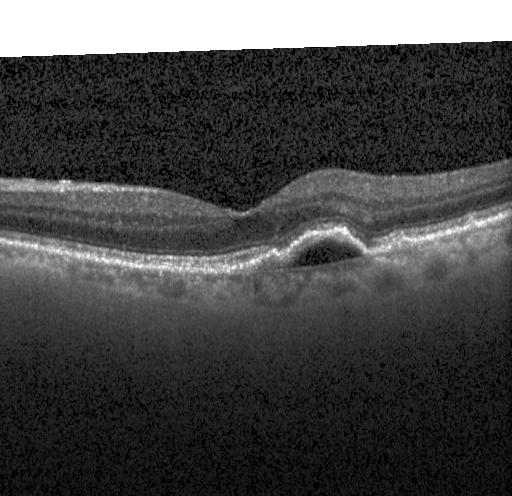 Dx: CNV.